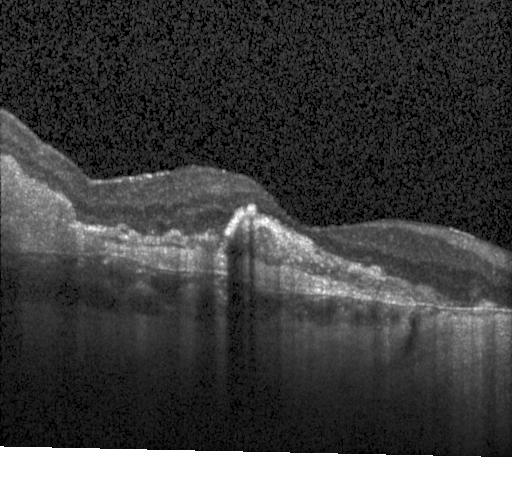
Retinal OCT B-scan.
Dx: a choroidal neovascular membrane.